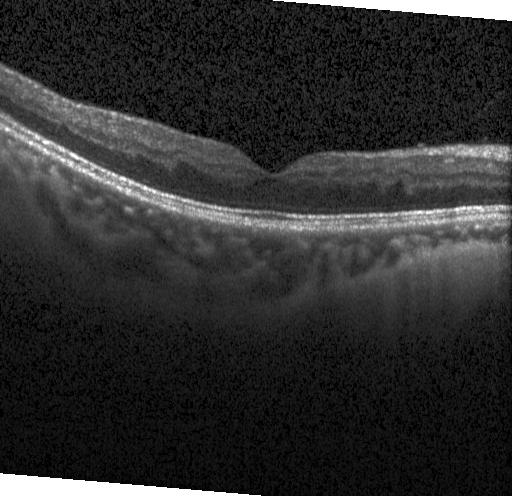 Heidelberg Spectralis OCT system, fovea-centered, optical coherence tomography scan, spectral-domain optical coherence tomography
Macular OCT: no choroidal neovascularization, diabetic macular edema, or drusen.